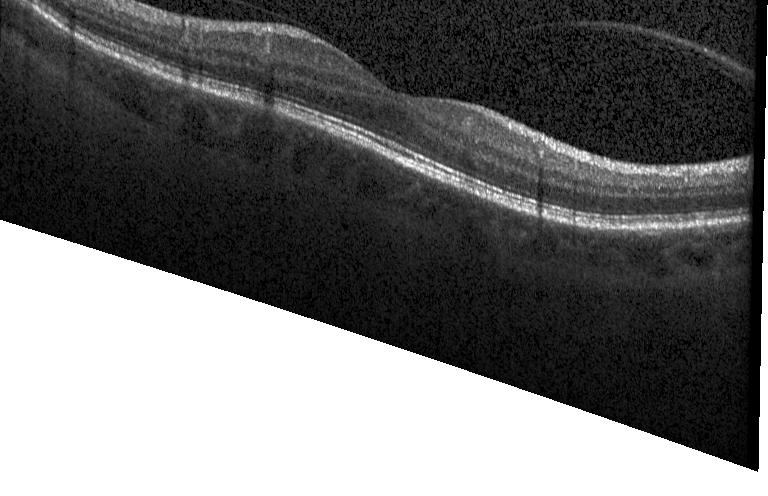

OCT scan showing no choroidal neovascularization, no diabetic macular edema, and no drusen.